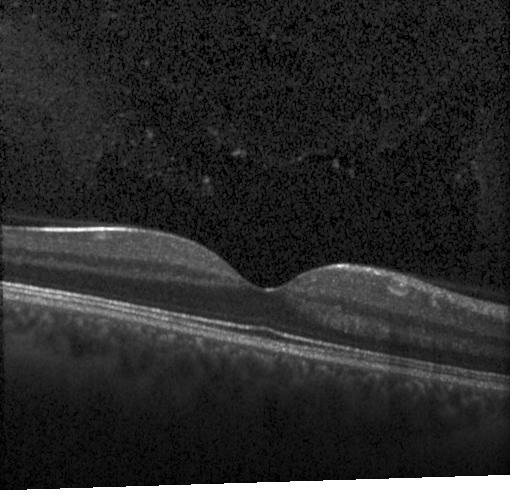 OCT scan showing no CNV, DME, or drusen.